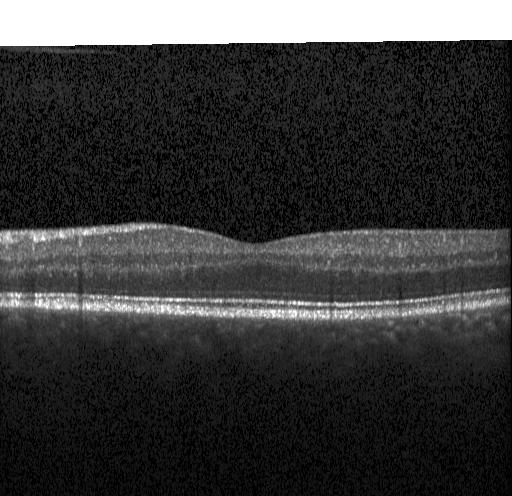 OCT B-scan · fovea-centered.
Finding: neither CNV, DME, nor drusen.